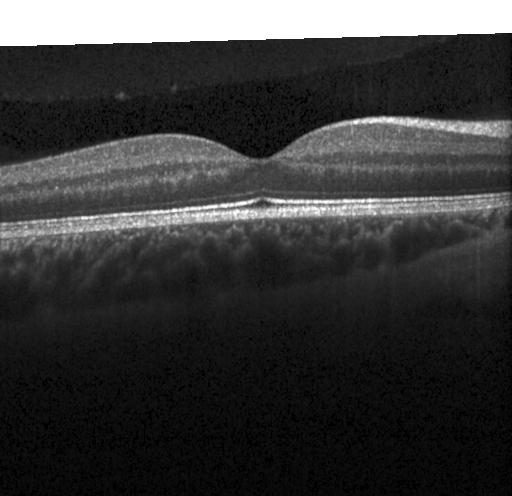

SD-OCT, Heidelberg Spectralis OCT system, fovea-centered, OCT B-scan
No CNV, no DME, and no drusen.